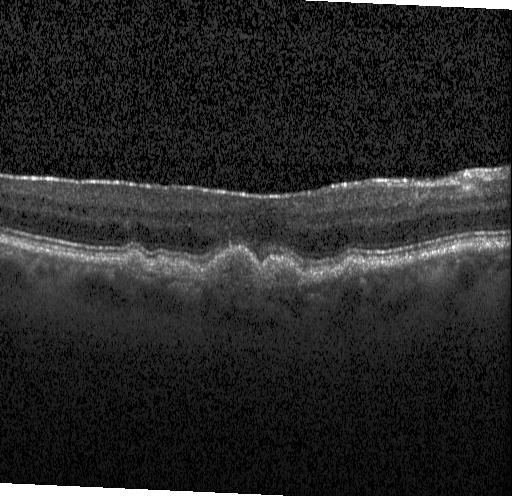
Through the macula; optical coherence tomography B-scan. Diagnosis: multiple drusen.